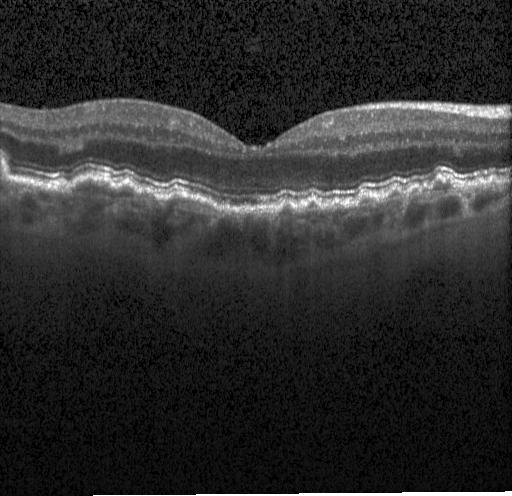
Dx: sub-RPE drusenoid deposits.